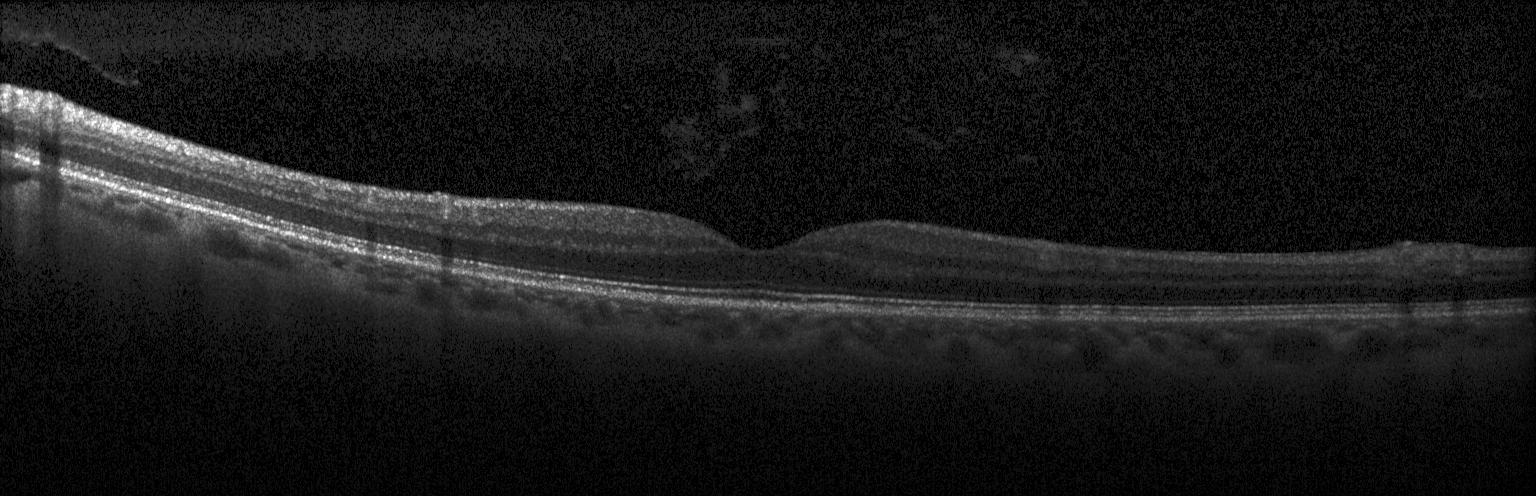
Spectral-domain optical coherence tomography; retinal OCT B-scan.
Dx: no choroidal neovascularization, diabetic macular edema, or drusen.